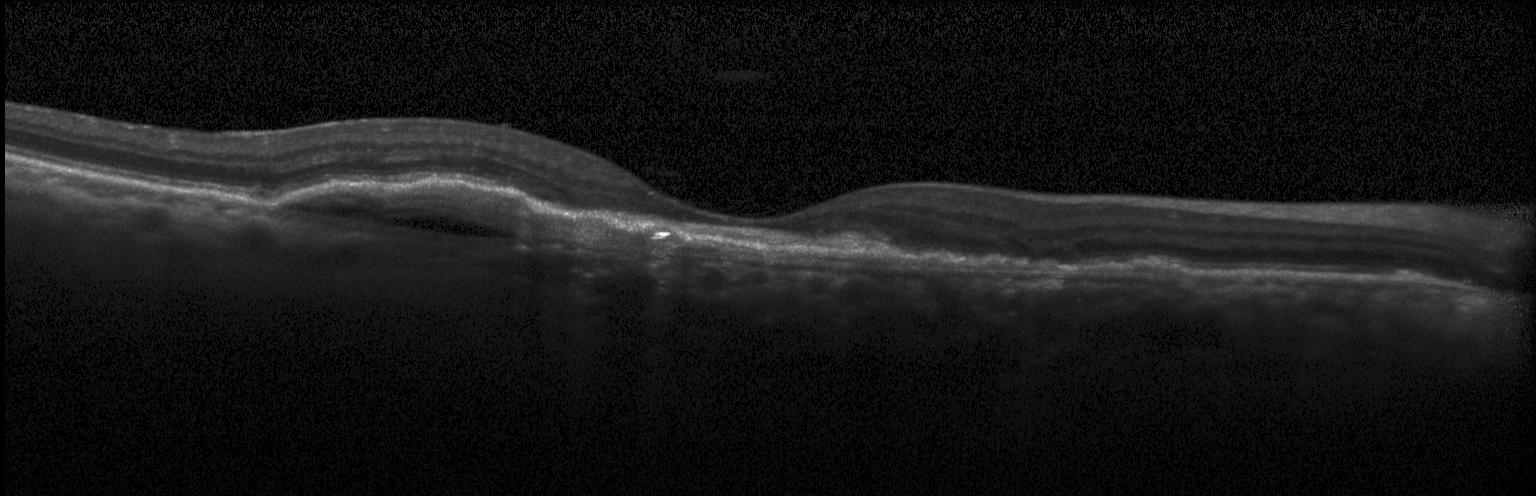 Diagnosis: a choroidal neovascular membrane.